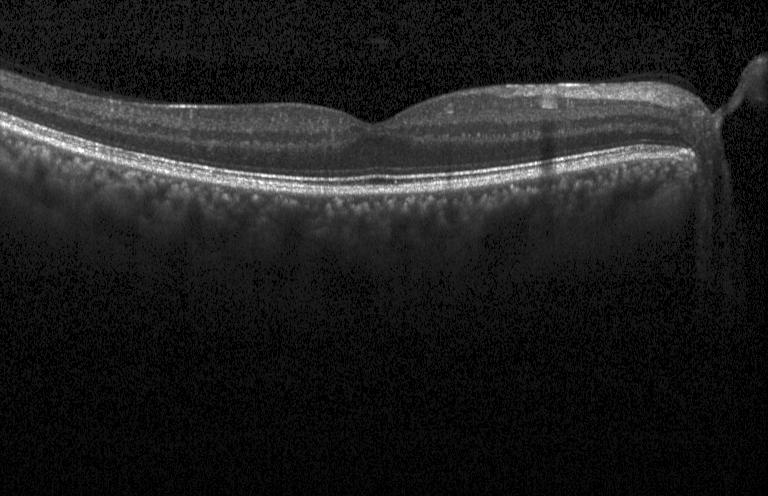
OCT finding: neither CNV, DME, nor drusen.